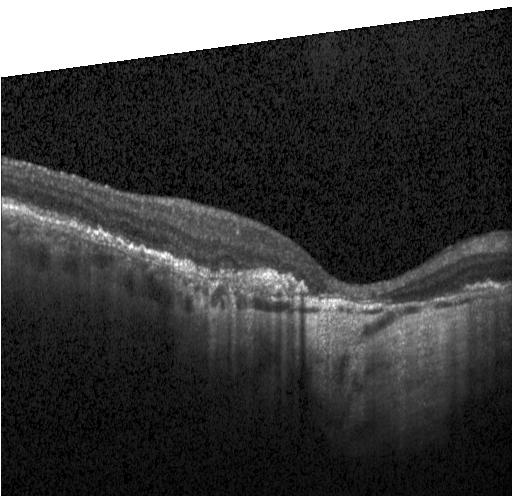

Instrument: Heidelberg Spectralis, through the macula, retinal OCT B-scan, spectral-domain optical coherence tomography — Impression: CNV.